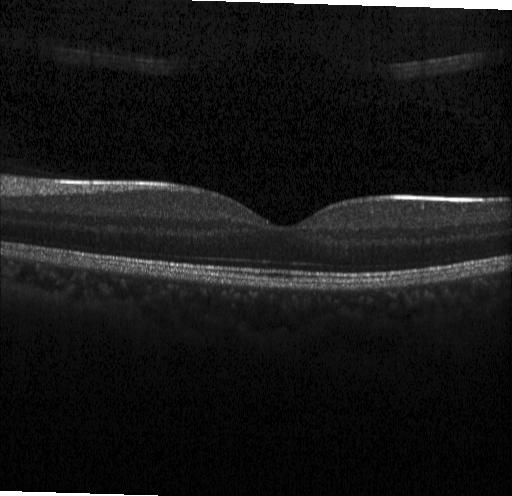 Dx: no evidence of CNV, DME, or drusen.